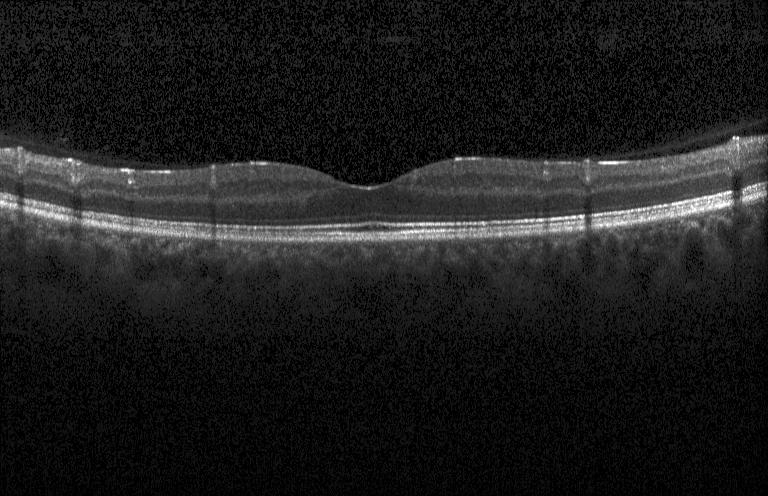 Through the macula, spectral-domain optical coherence tomography, OCT line scan, instrument: Heidelberg Spectralis — Dx: no evidence of choroidal neovascularization, diabetic macular edema, or drusen.